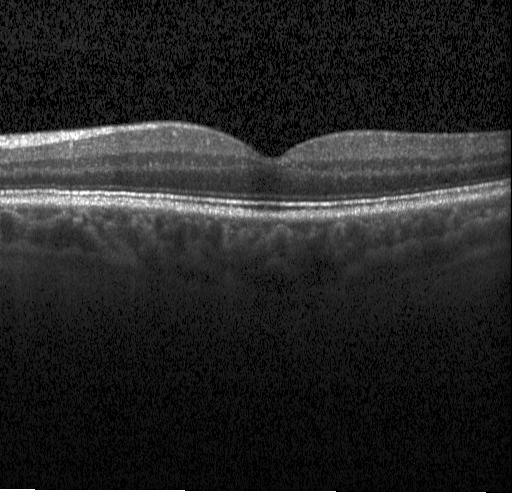
Spectral-domain optical coherence tomography · OCT line scan · through the macula
Diagnosis: neither choroidal neovascularization, diabetic macular edema, nor drusen.